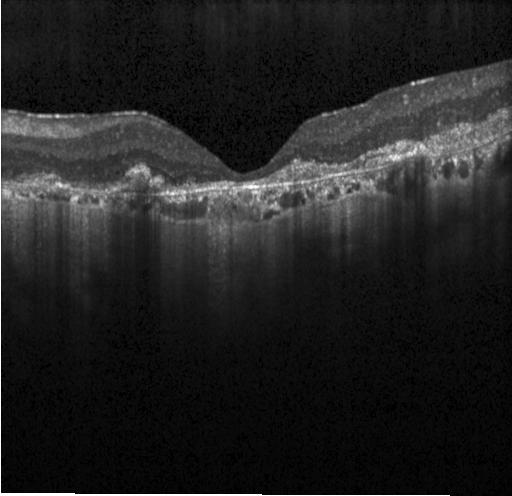 Retinal OCT cross-section; horizontal scan through the fovea; Heidelberg Spectralis OCT system. Dx: choroidal neovascularization (CNV).